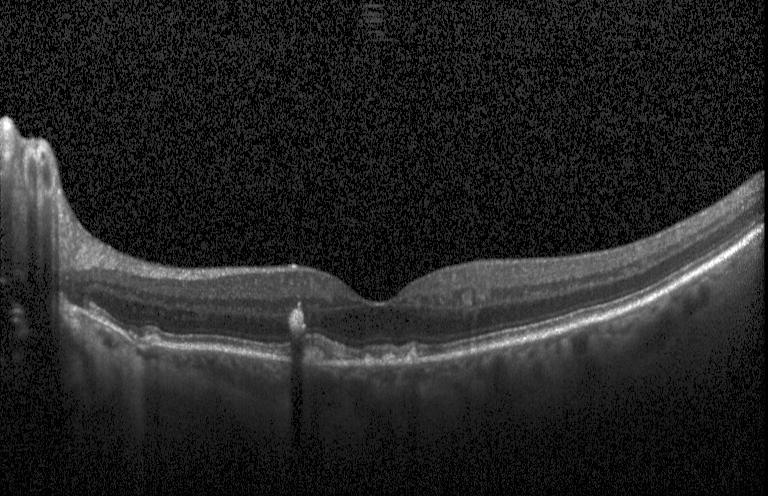 Macular OCT demonstrating sub-RPE drusenoid deposits.